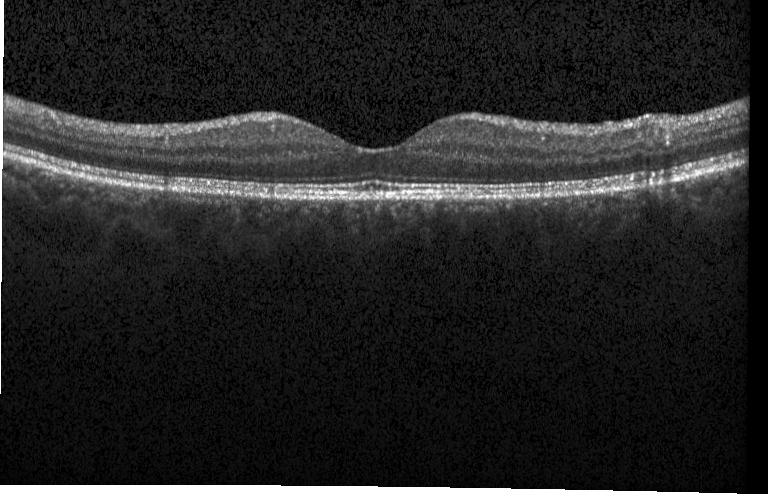 Macular scan, OCT line scan, SD-OCT, Heidelberg Spectralis OCT system
Finding: no evidence of choroidal neovascularization, diabetic macular edema, or drusen.